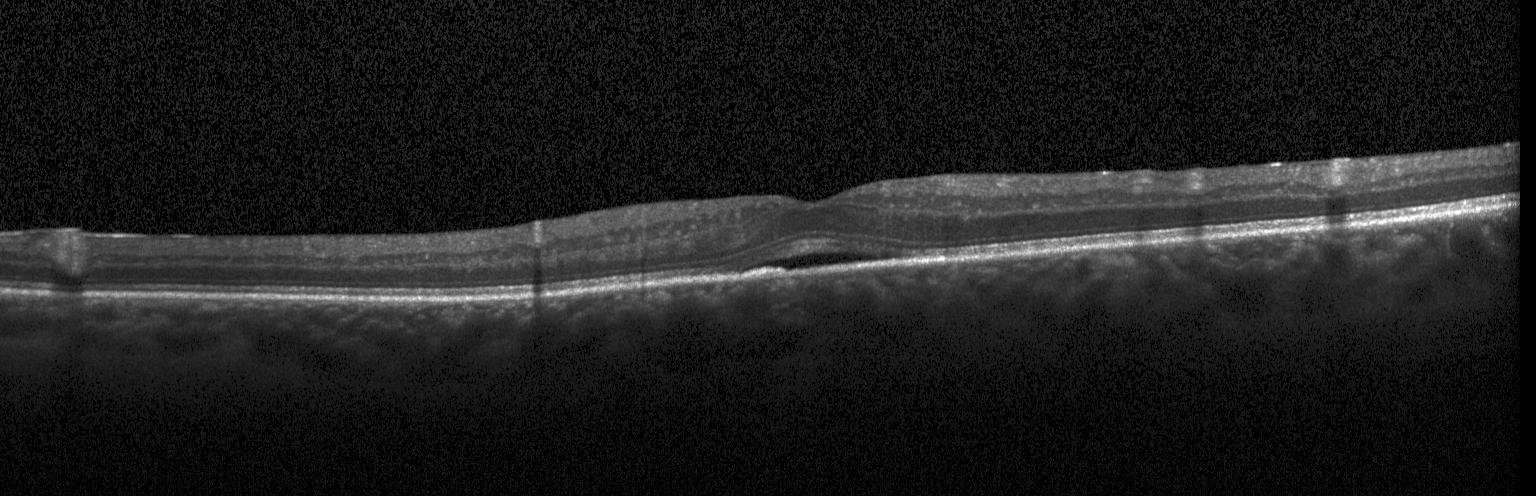

Assessment: choroidal neovascularization (CNV).